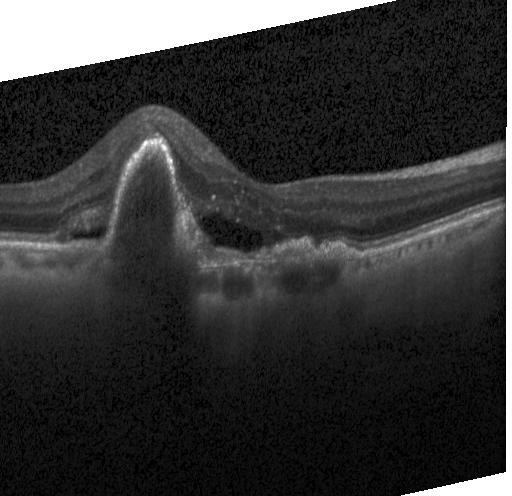 Optical coherence tomography B-scan.
This B-scan demonstrates a choroidal neovascular membrane.